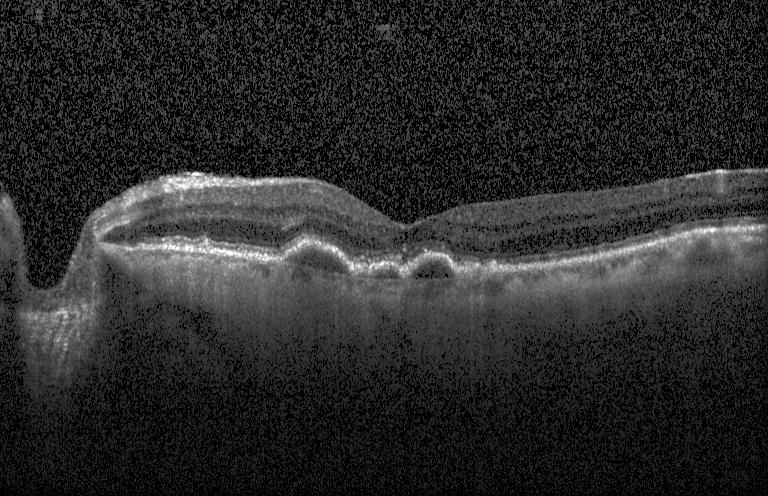

Optical coherence tomography scan. Centered on the fovea.
This B-scan demonstrates a choroidal neovascular membrane.